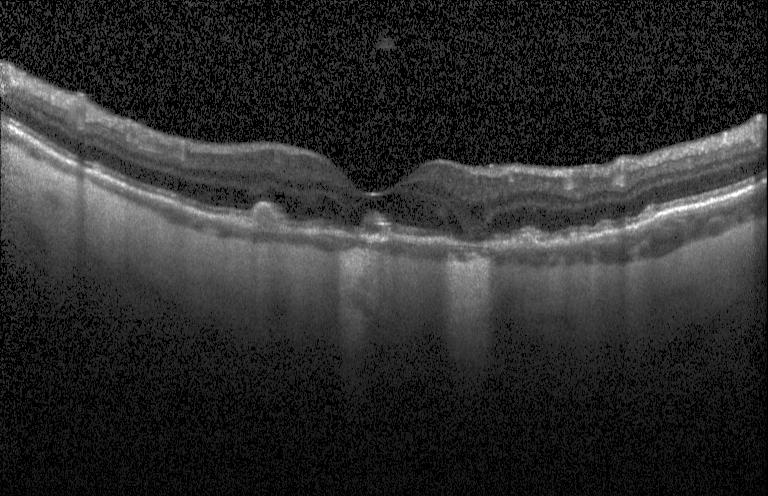 Heidelberg Spectralis. SD-OCT. Macular scan. Optical coherence tomography B-scan. Diagnosis: choroidal neovascularization.